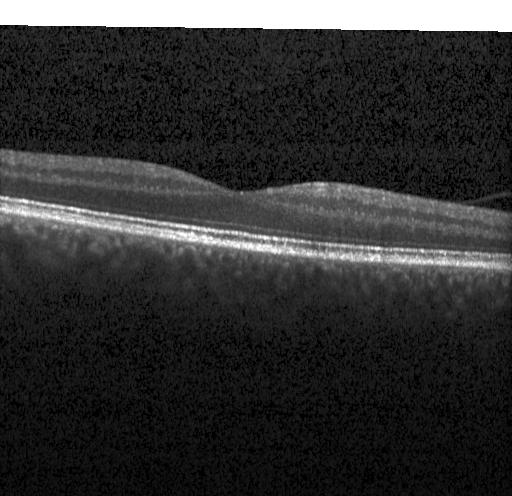

Instrument: Heidelberg Spectralis; spectral-domain optical coherence tomography; retinal OCT B-scan; macular scan
No choroidal neovascularization, diabetic macular edema, or drusen.